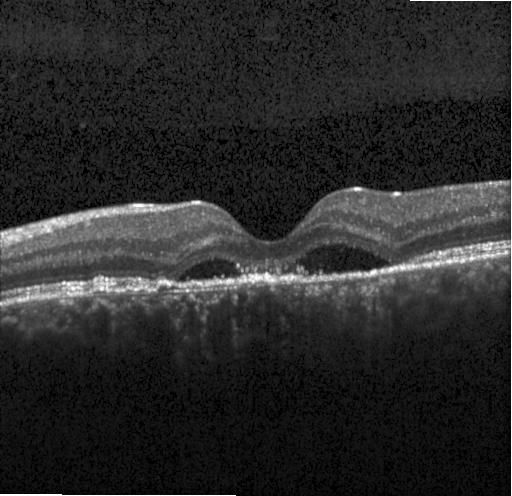

Diagnosis: a choroidal neovascular membrane.